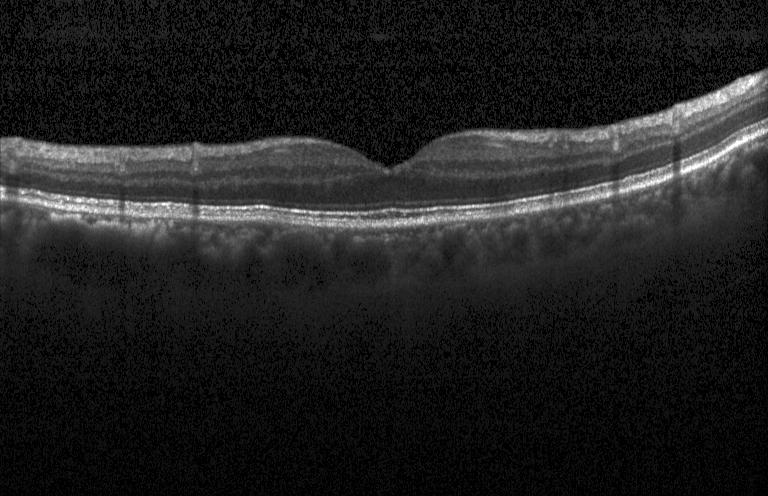
Macular OCT: no CNV, DME, or drusen.